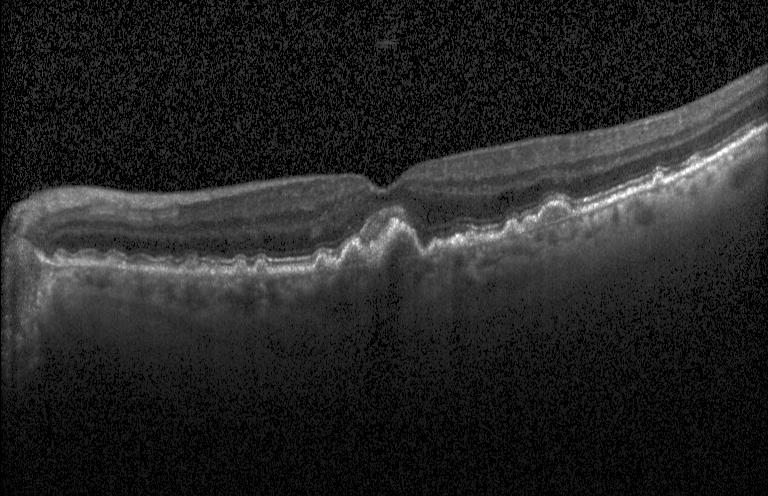 Assessment: CNV.